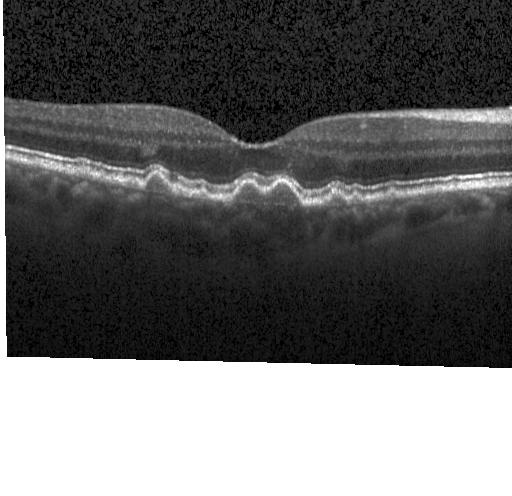
Finding: multiple drusen.